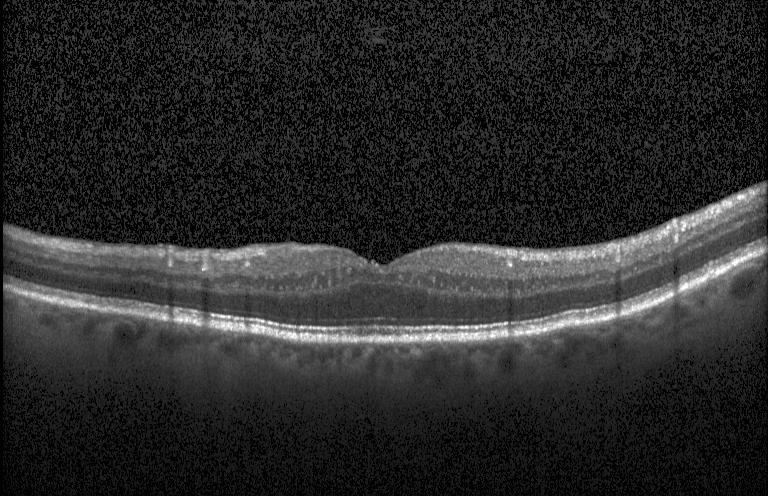
This B-scan demonstrates neither choroidal neovascularization, diabetic macular edema, nor drusen.